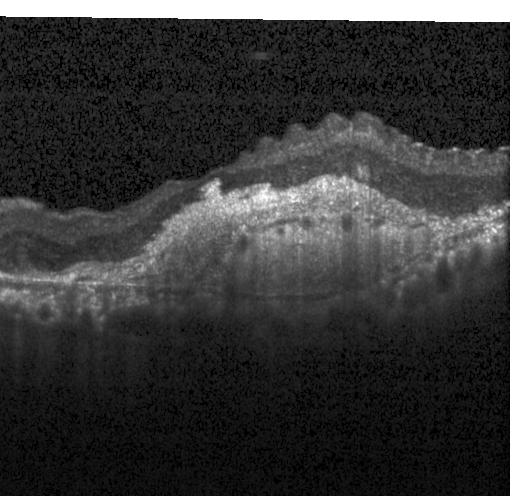

Assessment: CNV.